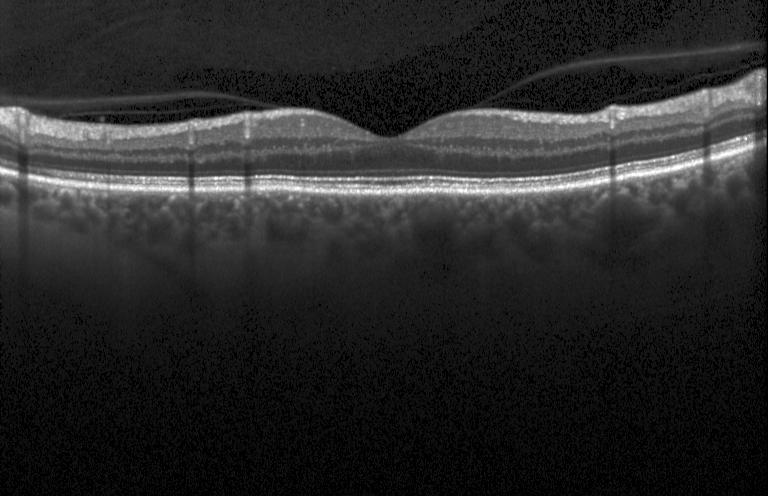

Heidelberg Spectralis · OCT B-scan. Macular OCT: no CNV, no DME, and no drusen.